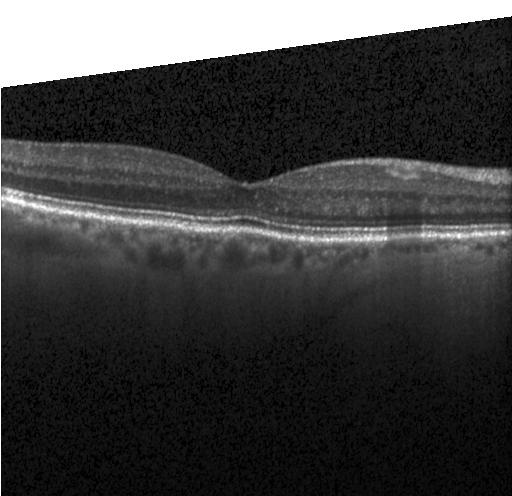

Optical coherence tomography B-scan, acquired on a Heidelberg Spectralis
Diagnosis: no evidence of choroidal neovascularization, diabetic macular edema, or drusen.